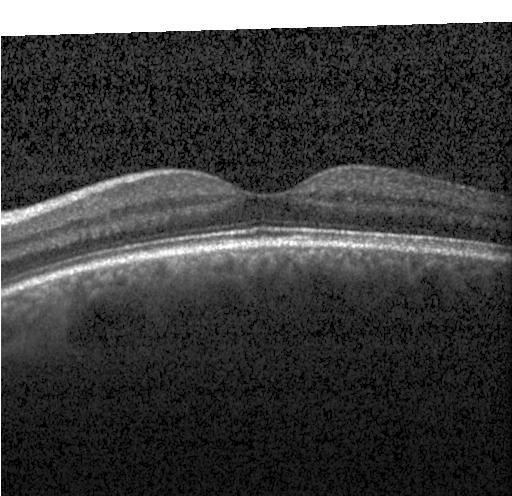 OCT B-scan · SD-OCT · macular scan.
Diagnosis: no evidence of CNV, DME, or drusen.